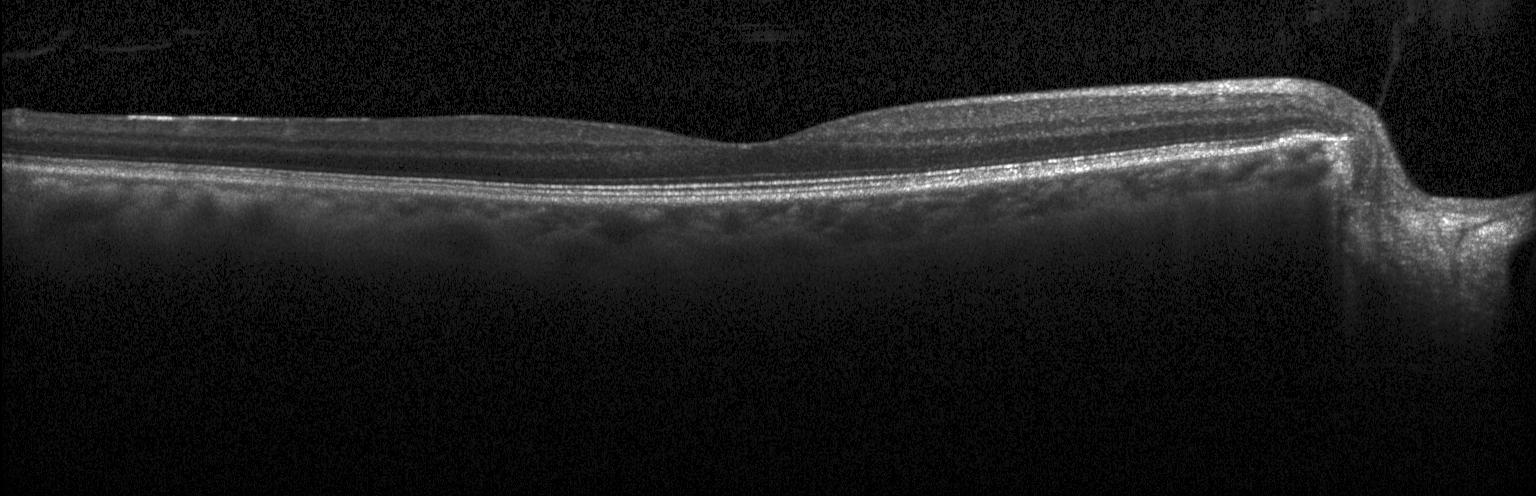
Spectral-domain optical coherence tomography, retinal OCT B-scan — The scan shows neither CNV, DME, nor drusen.